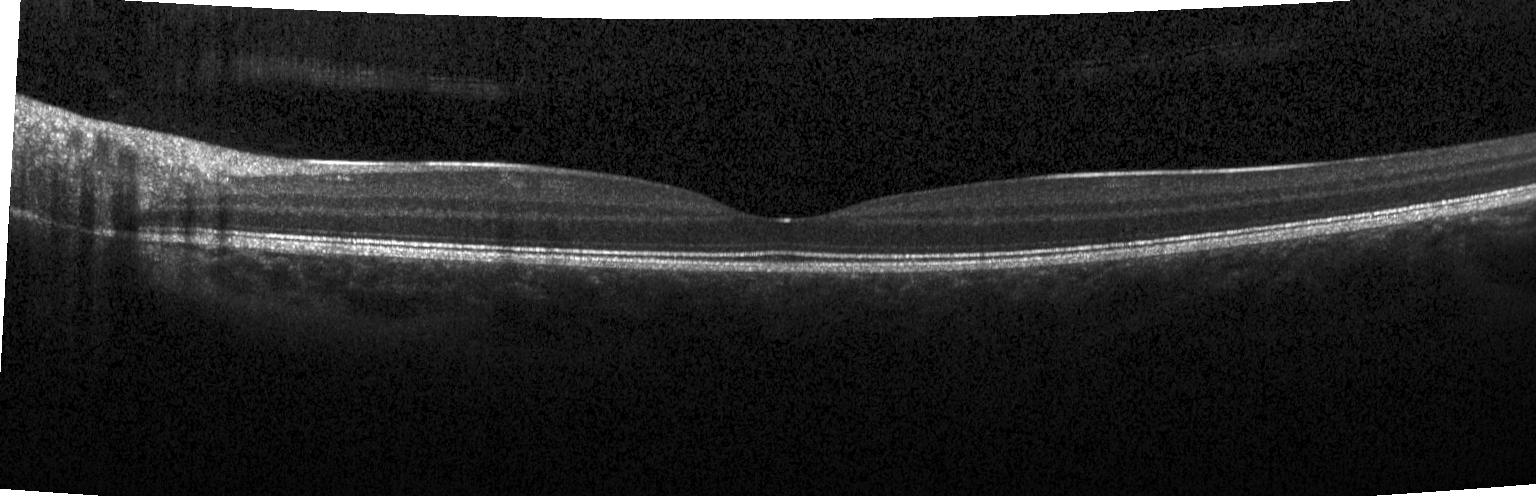
OCT B-scan showing neither CNV, DME, nor drusen.